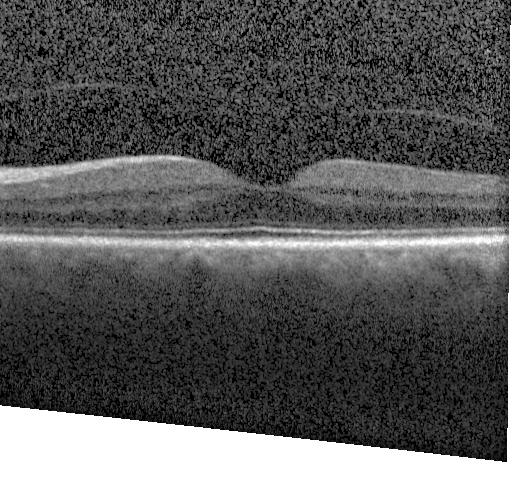

Instrument: Heidelberg Spectralis · optical coherence tomography scan · horizontal scan through the fovea · spectral-domain OCT.
Dx: no choroidal neovascularization, diabetic macular edema, or drusen.